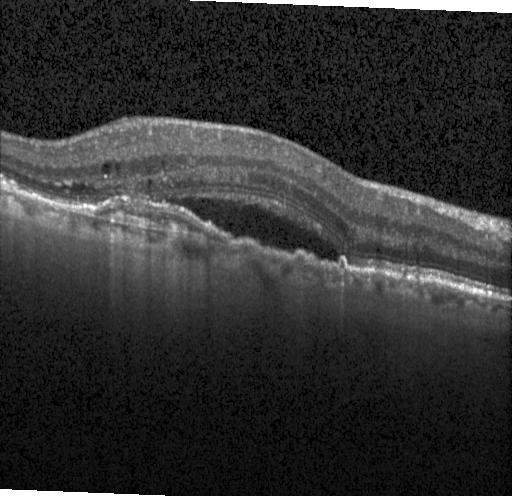

Finding: choroidal neovascularization.